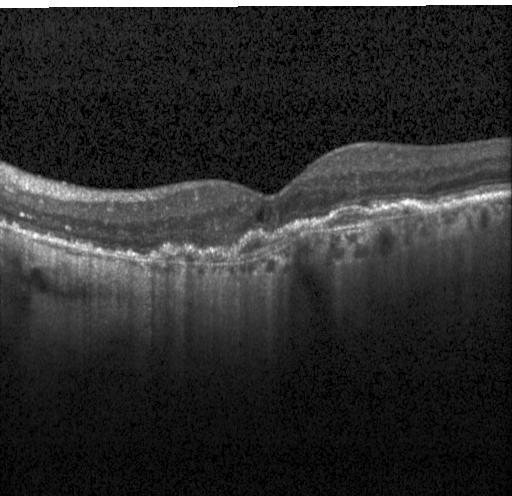
Finding: a choroidal neovascular membrane.